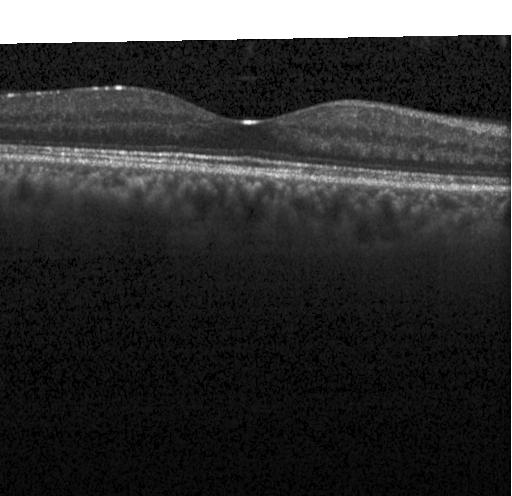
Optical coherence tomography B-scan.
Diagnosis: neither choroidal neovascularization, diabetic macular edema, nor drusen.